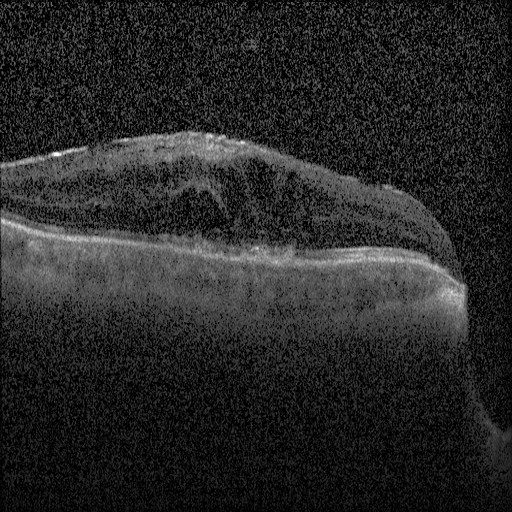

Optical coherence tomography B-scan.
OCT finding: diabetic macular edema (DME).